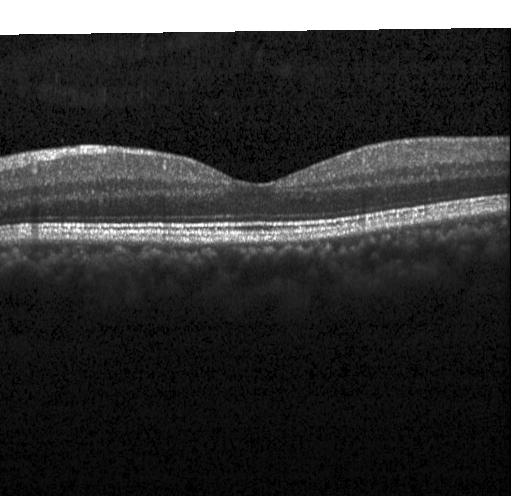
Acquired on a Heidelberg Spectralis, retinal OCT B-scan, spectral-domain OCT — Finding: no choroidal neovascularization, no diabetic macular edema, and no drusen.